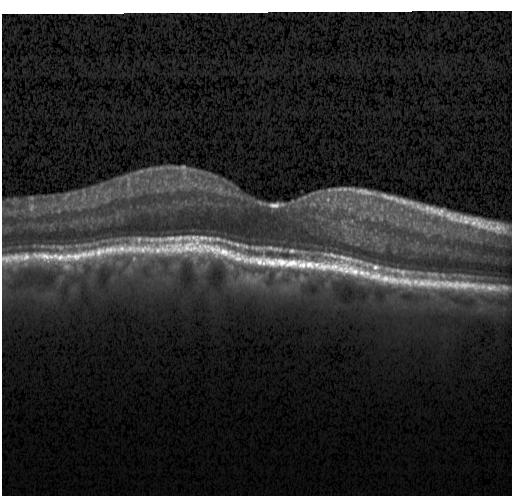 Retinal OCT cross-section. OCT finding: no CNV, DME, or drusen.